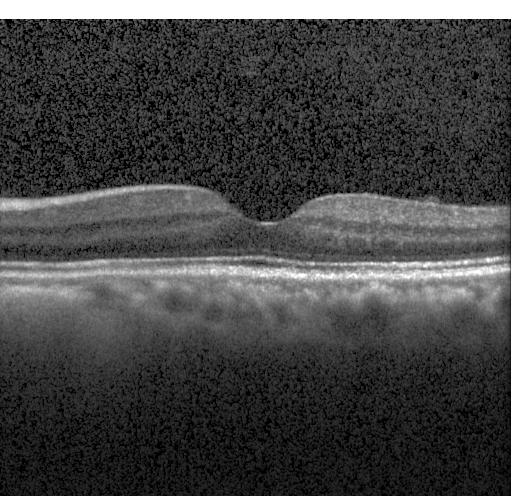 No choroidal neovascularization, diabetic macular edema, or drusen.